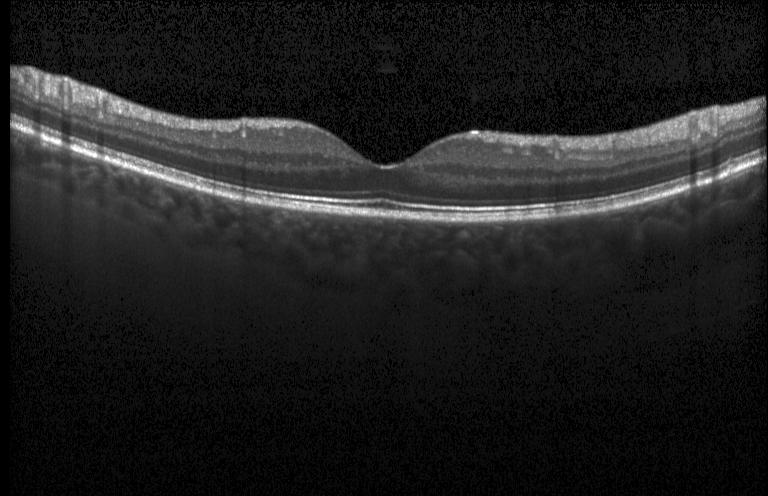

Macular OCT: neither choroidal neovascularization, diabetic macular edema, nor drusen.